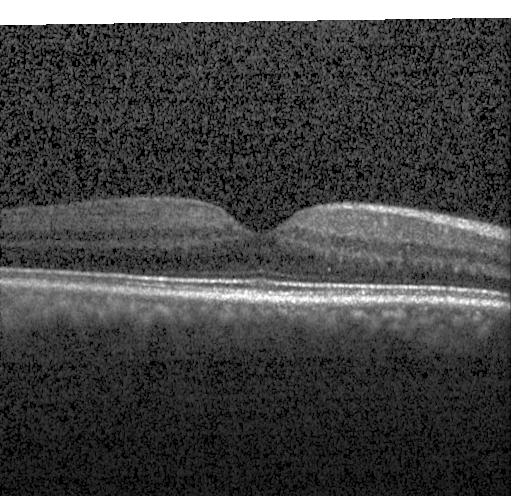

No evidence of CNV, DME, or drusen.